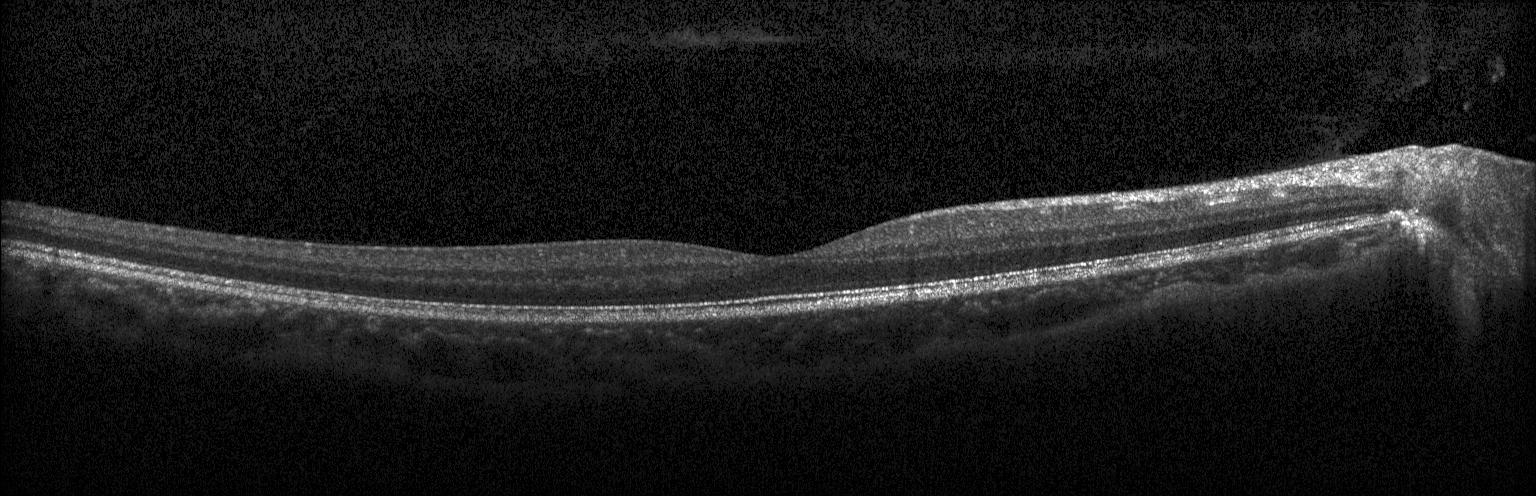 OCT line scan — The scan shows neither choroidal neovascularization, diabetic macular edema, nor drusen.